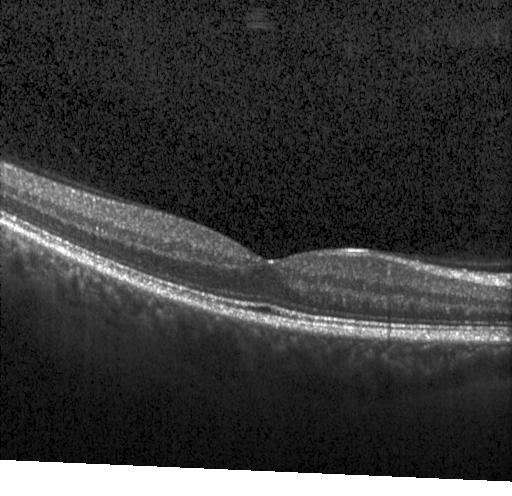

Impression: neither choroidal neovascularization, diabetic macular edema, nor drusen.